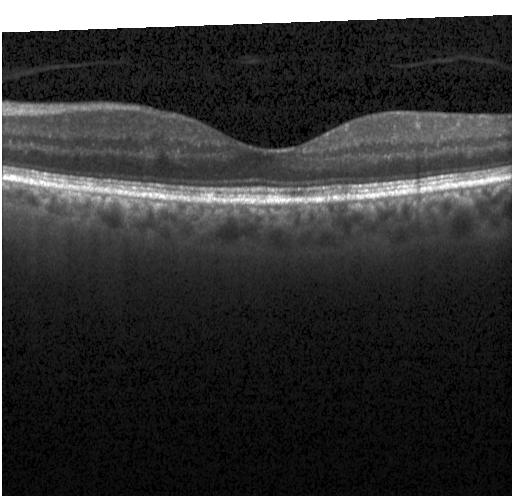
Finding: neither choroidal neovascularization, diabetic macular edema, nor drusen.